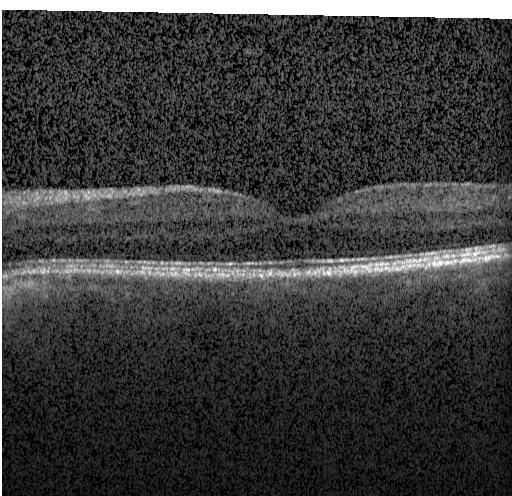

Retinal OCT cross-section. Diagnosis: no evidence of CNV, DME, or drusen.